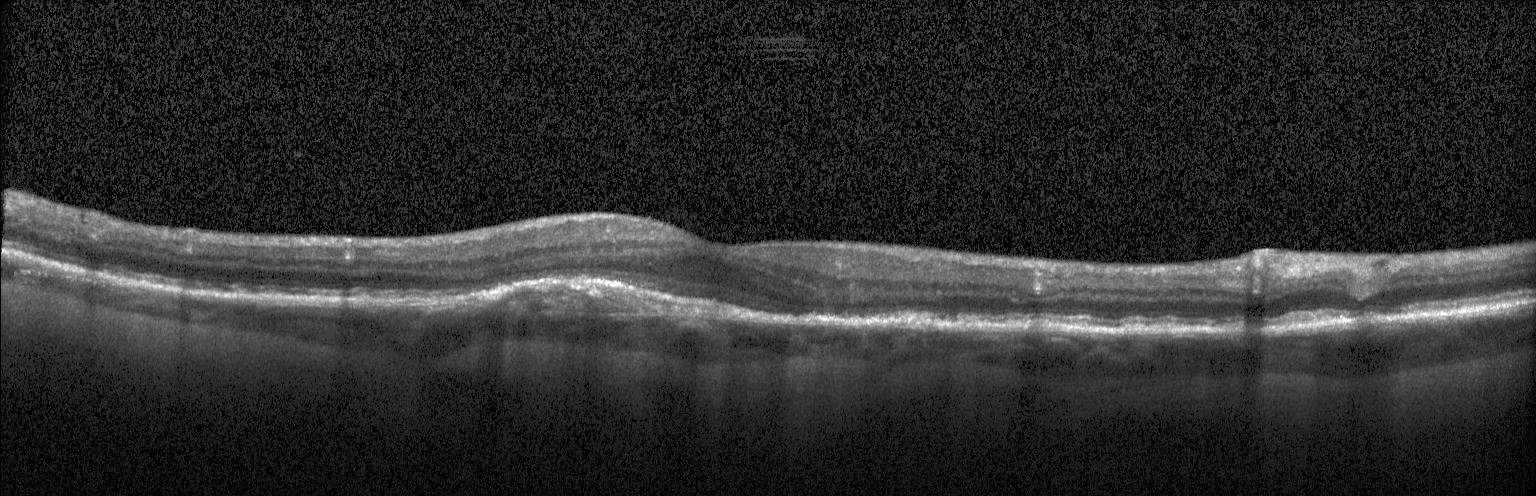 Assessment: a choroidal neovascular membrane.